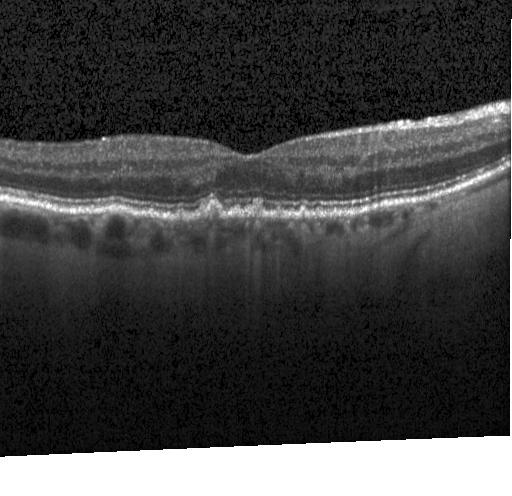 Heidelberg Spectralis OCT system. Macular scan. Spectral-domain OCT. Optical coherence tomography scan.
Finding: sub-RPE drusenoid deposits.